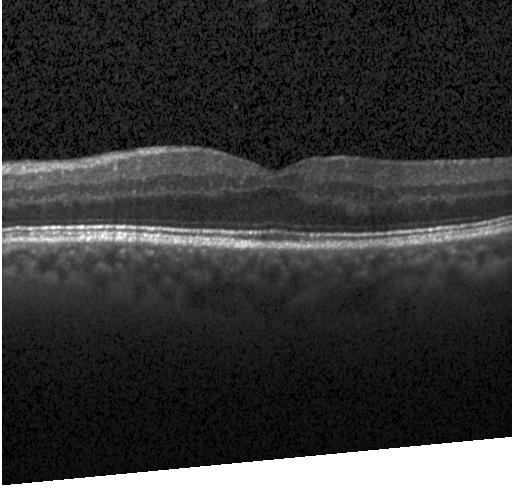
Impression: neither CNV, DME, nor drusen.